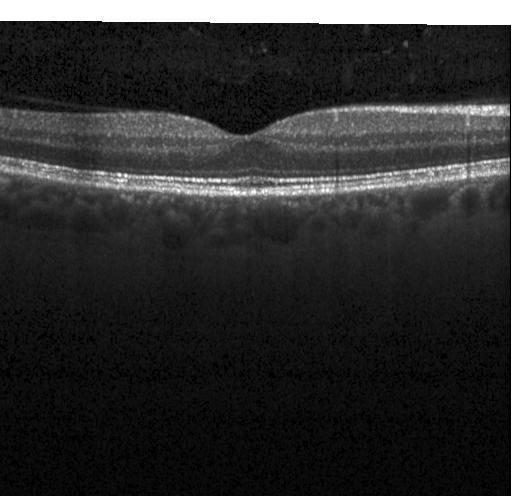 OCT finding: neither choroidal neovascularization, diabetic macular edema, nor drusen.